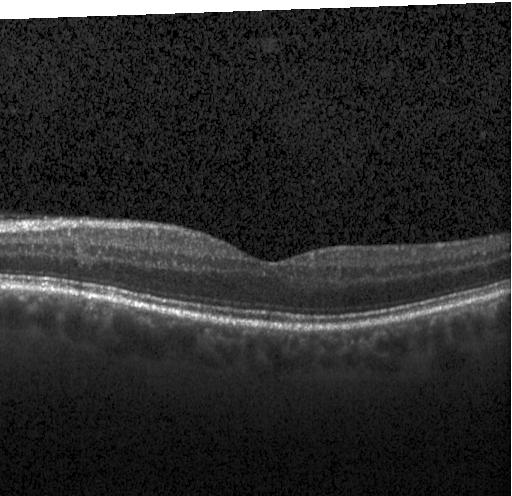

Macular OCT: no CNV, no DME, and no drusen.